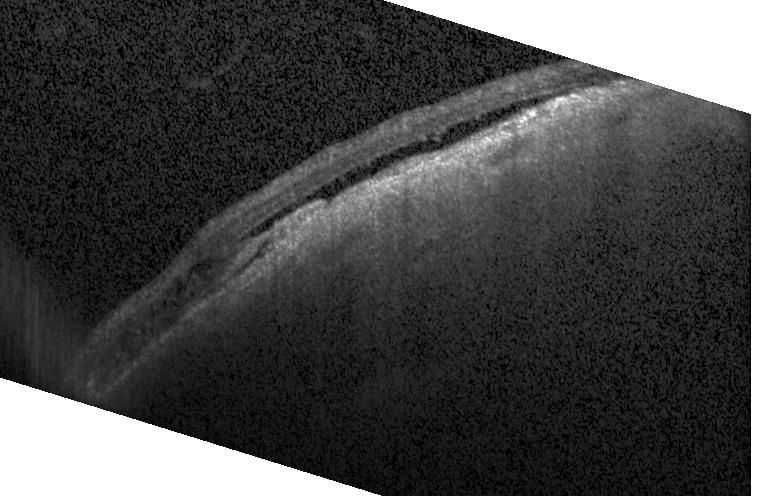
Impression: CNV.